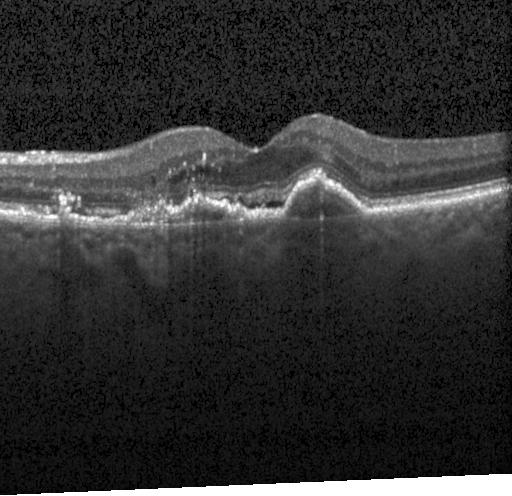 OCT B-scan.
Assessment: choroidal neovascularization (CNV).